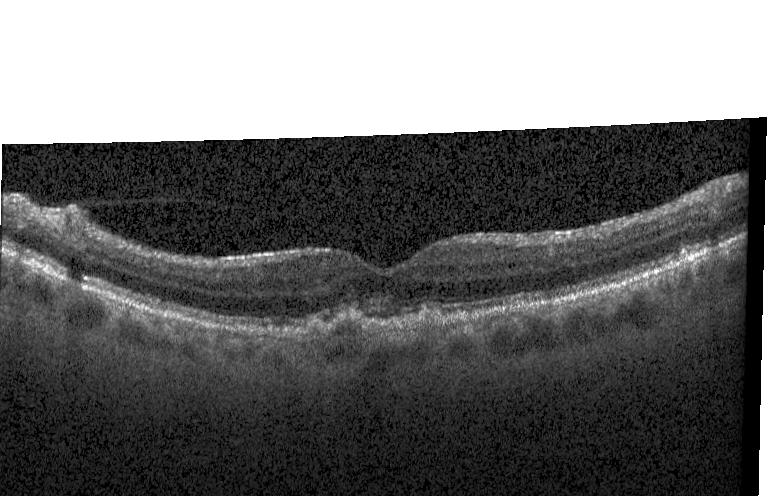 Retinal OCT cross-section · Heidelberg Spectralis
A choroidal neovascular membrane.